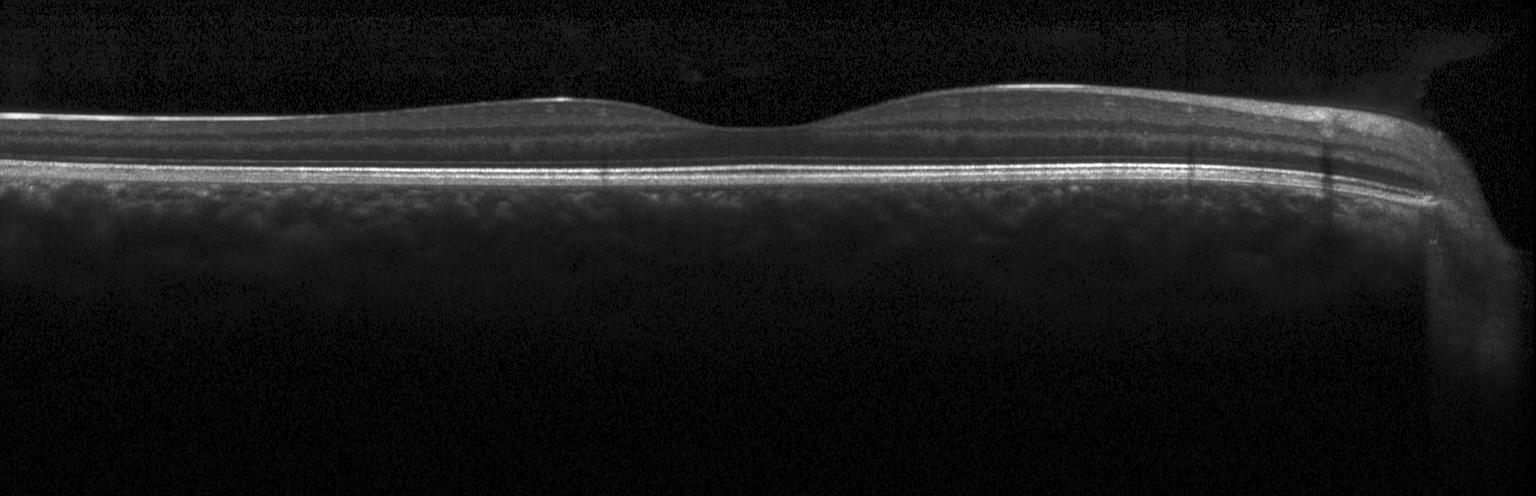
OCT line scan. Diagnosis: no choroidal neovascularization, no diabetic macular edema, and no drusen.